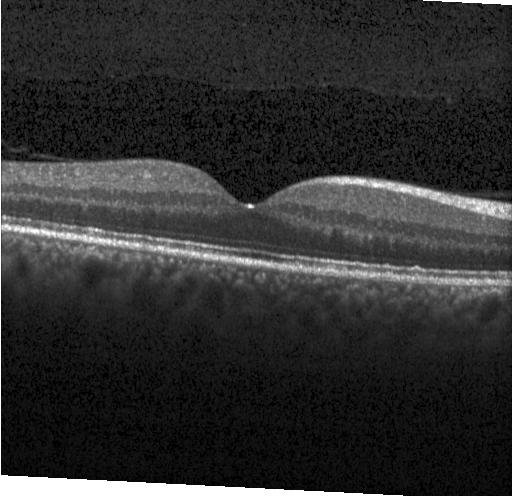
OCT line scan · centered on the fovea
The scan shows no choroidal neovascularization, diabetic macular edema, or drusen.